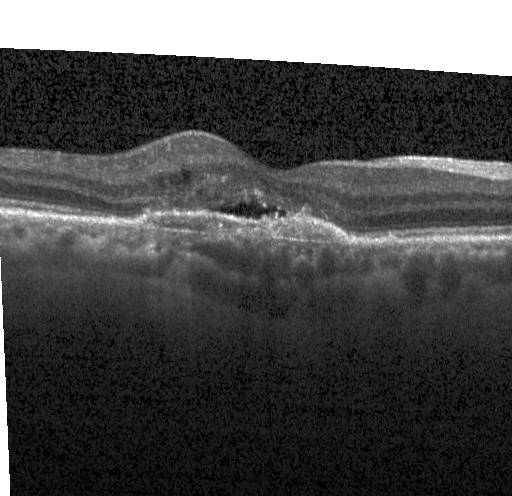

Dx: choroidal neovascularization (CNV).